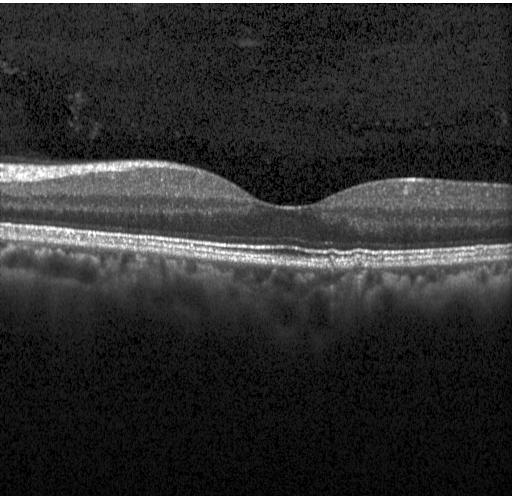

OCT finding: drusen.